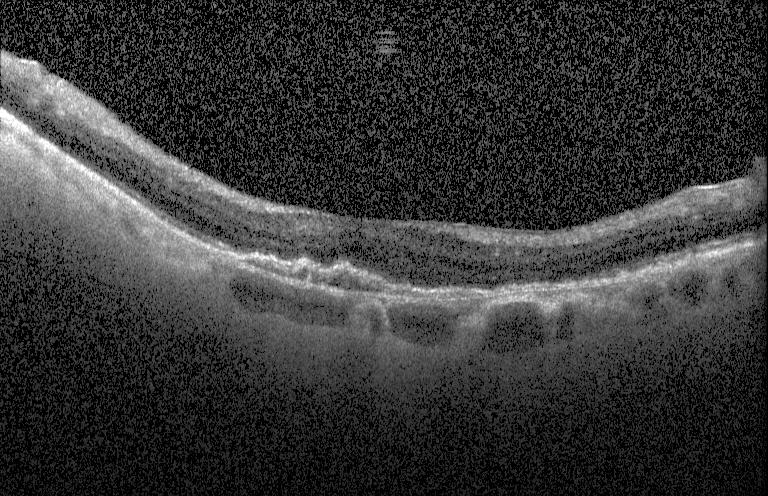

Assessment: a choroidal neovascular membrane.